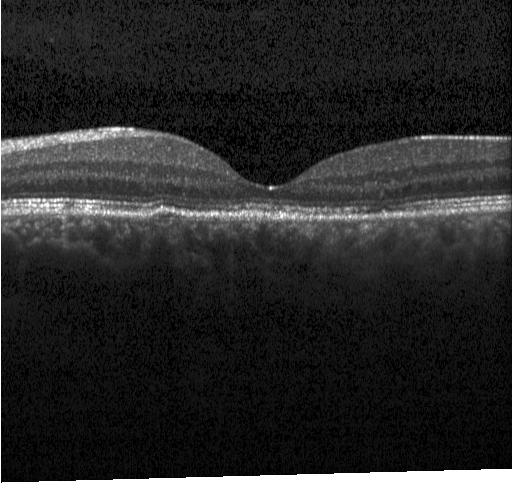

Optical coherence tomography scan.
Finding: multiple drusen.